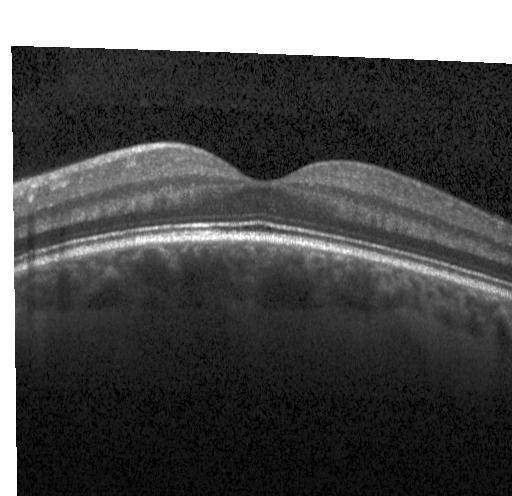

Macular scan. Optical coherence tomography B-scan. Spectral-domain OCT. Assessment: no choroidal neovascularization, no diabetic macular edema, and no drusen.